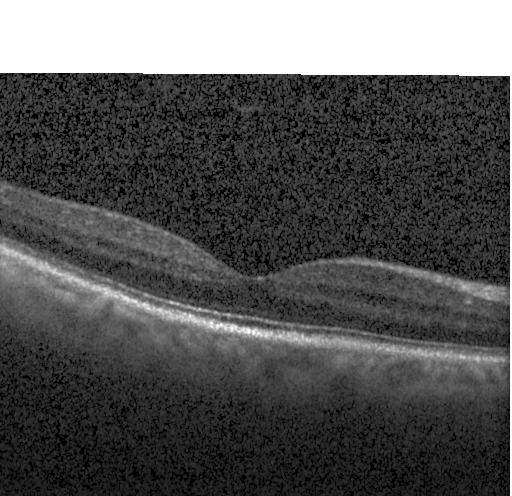
Retinal OCT cross-section showing neither CNV, DME, nor drusen.